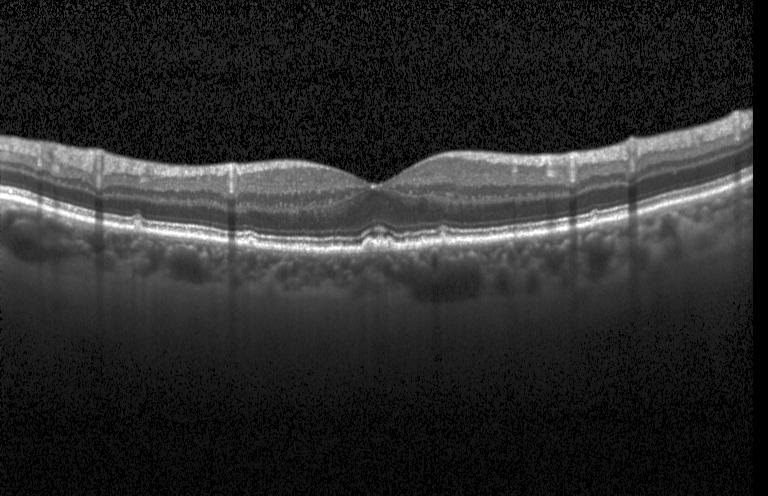 Heidelberg Spectralis OCT system. Retinal OCT cross-section — Assessment: sub-RPE drusenoid deposits.